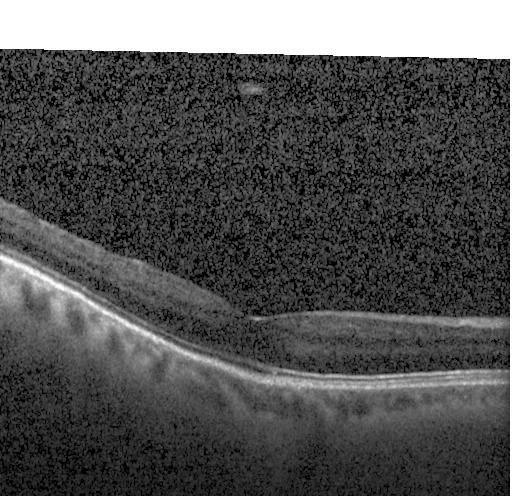

OCT line scan
Macular OCT: neither choroidal neovascularization, diabetic macular edema, nor drusen.